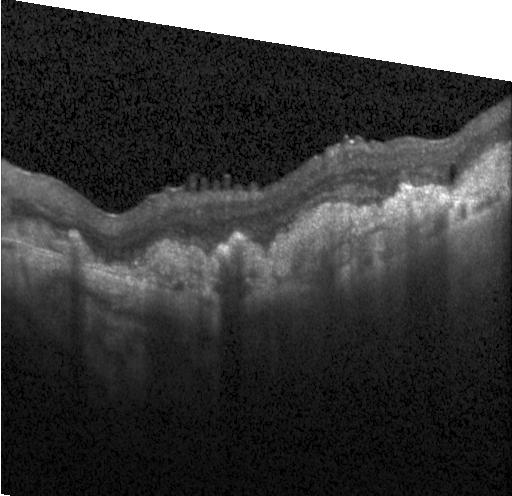

OCT scan showing choroidal neovascularization.